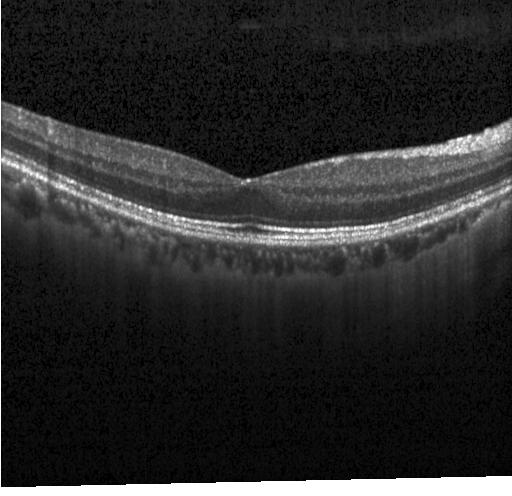 SD-OCT · through the macula · Heidelberg Spectralis OCT system · OCT B-scan.
Dx: neither CNV, DME, nor drusen.